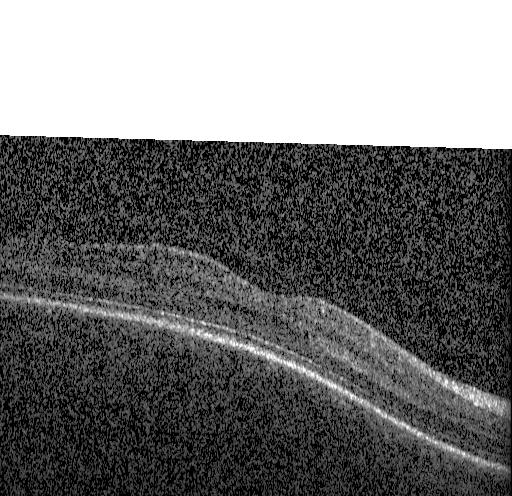
Optical coherence tomography B-scan · SD-OCT — This B-scan demonstrates no evidence of CNV, DME, or drusen.